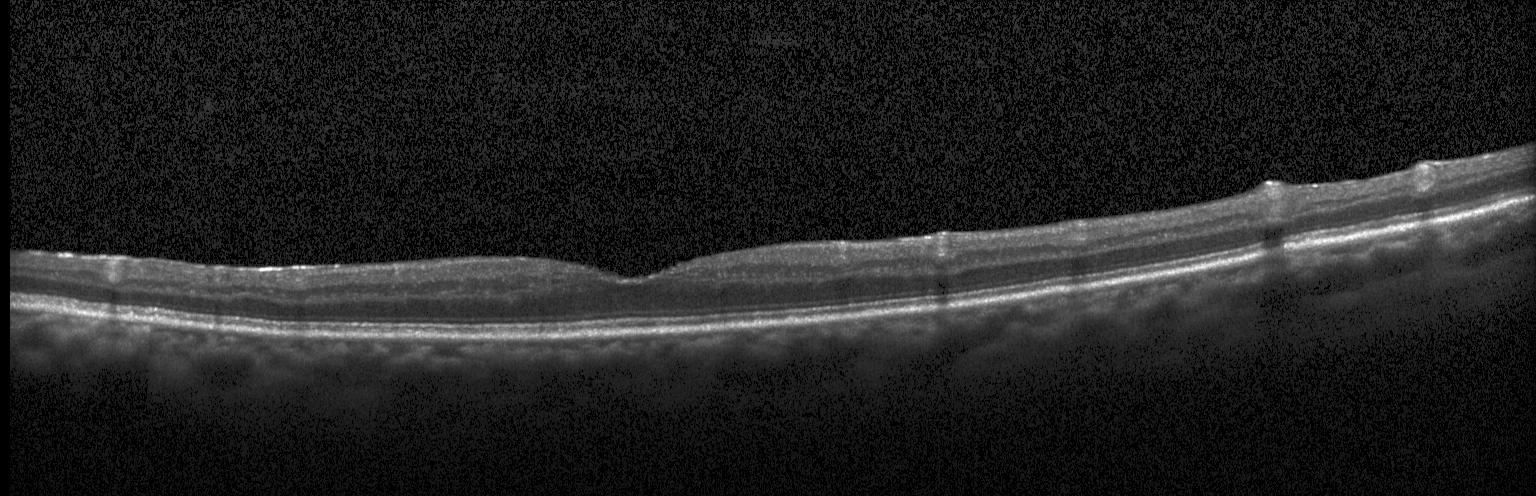

Diagnosis: no evidence of choroidal neovascularization, diabetic macular edema, or drusen.